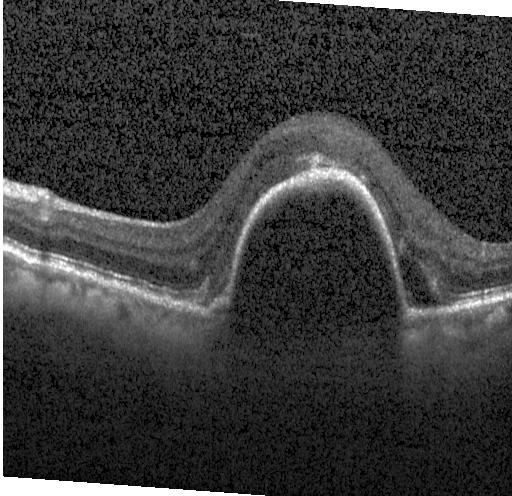 Fovea-centered. Optical coherence tomography scan. Heidelberg Spectralis.
OCT finding: choroidal neovascularization.